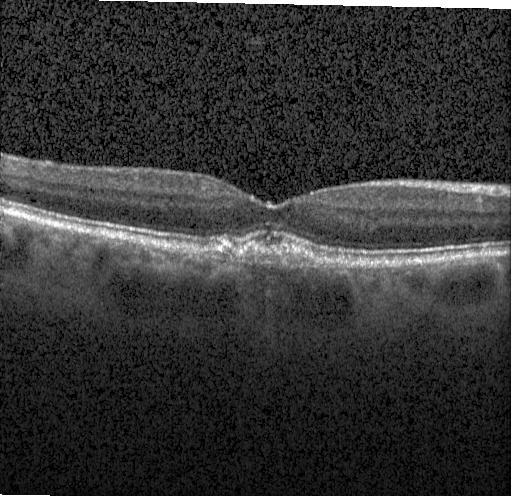
Assessment: drusen.